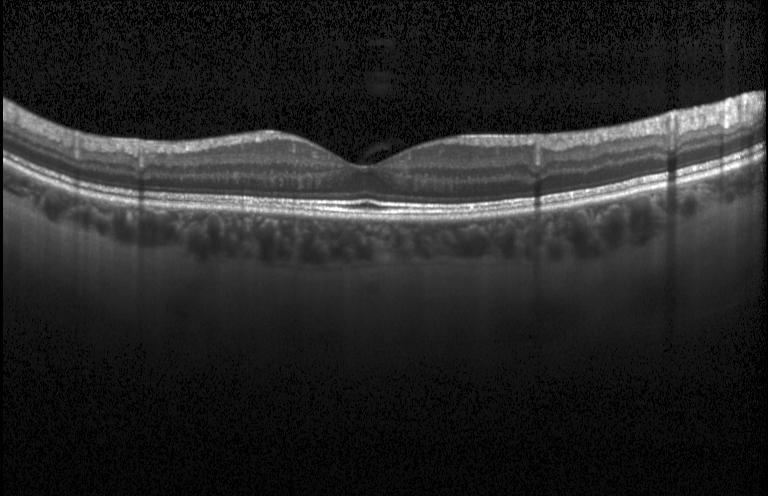

Optical coherence tomography B-scan
Assessment: no choroidal neovascularization, diabetic macular edema, or drusen.